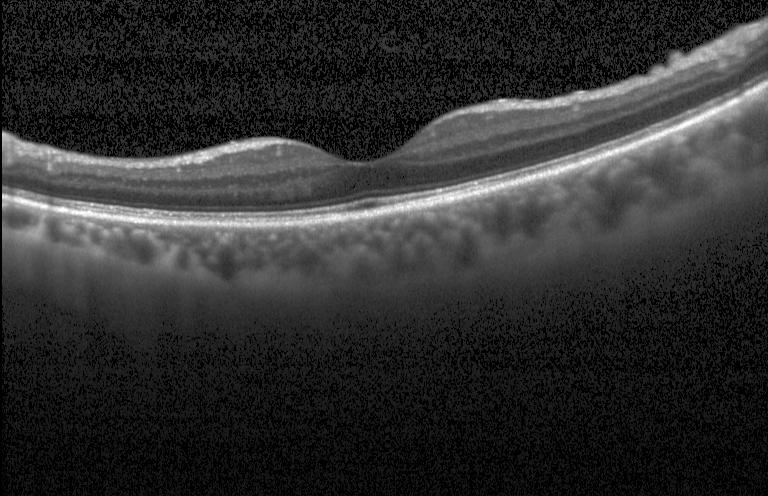
OCT B-scan showing neither choroidal neovascularization, diabetic macular edema, nor drusen.